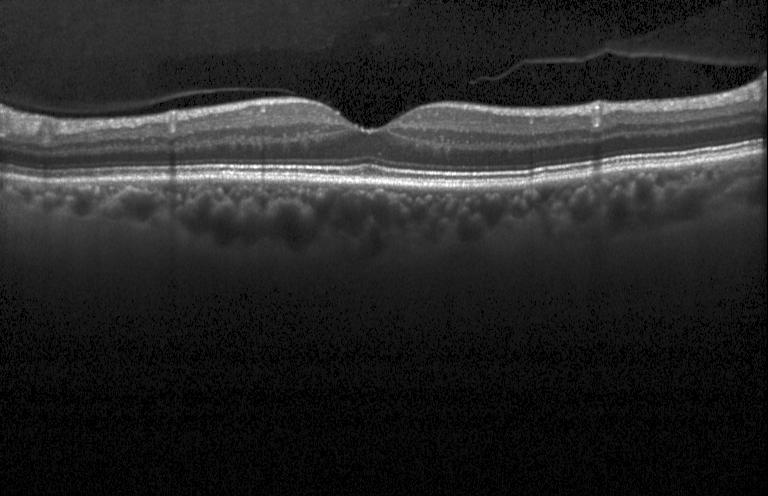
Impression: no choroidal neovascularization, no diabetic macular edema, and no drusen.